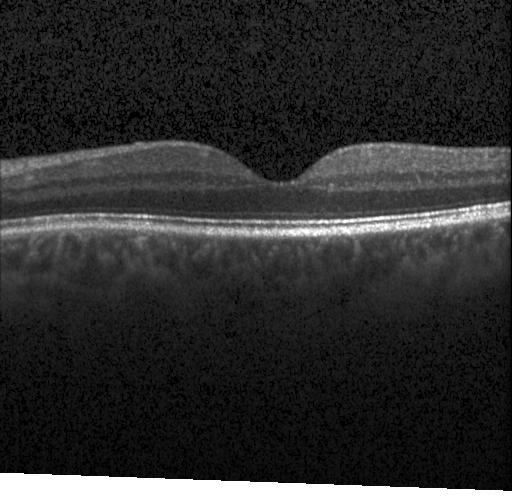 Acquired on a Heidelberg Spectralis, optical coherence tomography scan. Impression: neither choroidal neovascularization, diabetic macular edema, nor drusen.